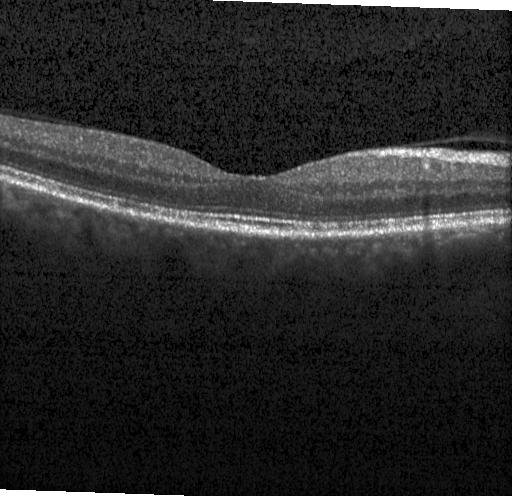

Heidelberg Spectralis · retinal OCT B-scan · spectral-domain OCT. Neither CNV, DME, nor drusen.